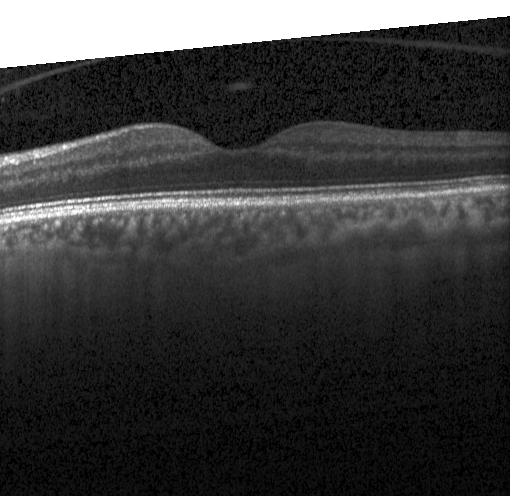

Spectral-domain optical coherence tomography. Centered on the fovea. Optical coherence tomography scan. Diagnosis: no choroidal neovascularization, diabetic macular edema, or drusen.